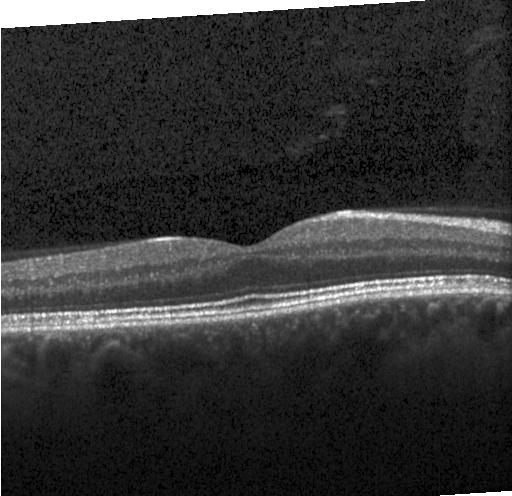 Spectral-domain optical coherence tomography, OCT line scan, horizontal scan through the fovea
OCT finding: no evidence of choroidal neovascularization, diabetic macular edema, or drusen.